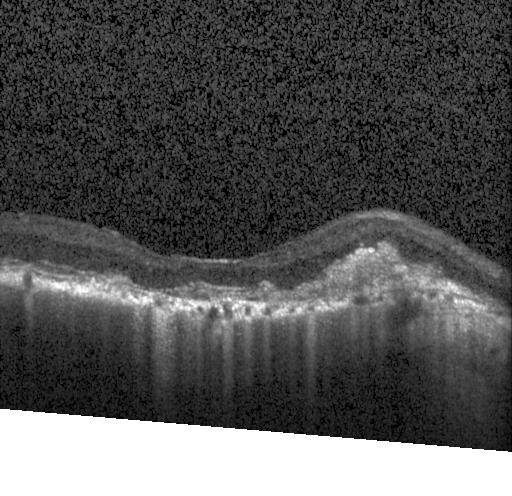
Optical coherence tomography scan; spectral-domain OCT.
Macular OCT: a choroidal neovascular membrane.